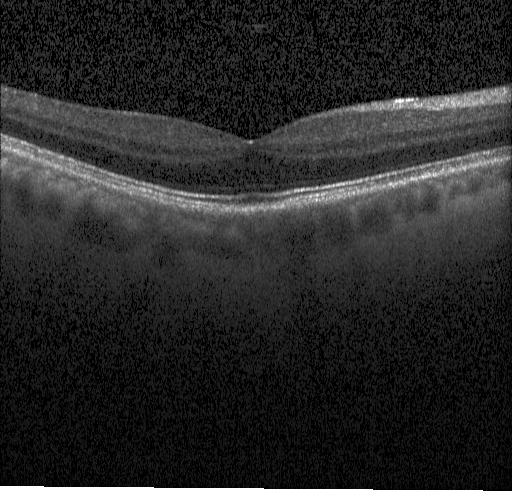 OCT finding: no choroidal neovascularization, no diabetic macular edema, and no drusen.